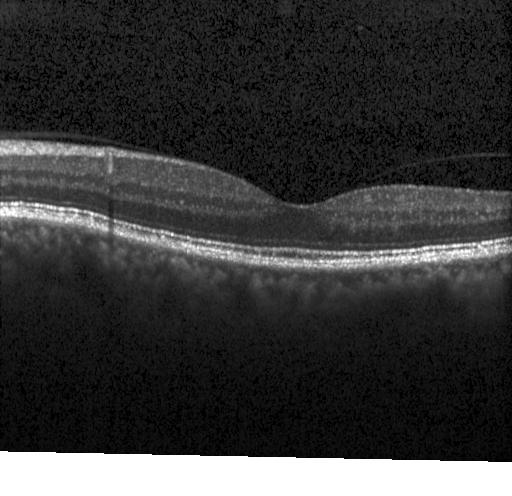

Spectral-domain optical coherence tomography; OCT line scan.
Finding: neither choroidal neovascularization, diabetic macular edema, nor drusen.